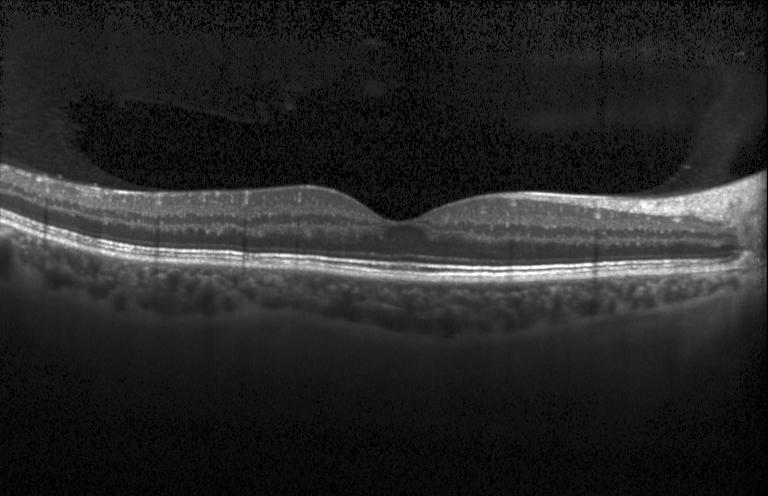

Retinal OCT B-scan — OCT finding: no CNV, no DME, and no drusen.